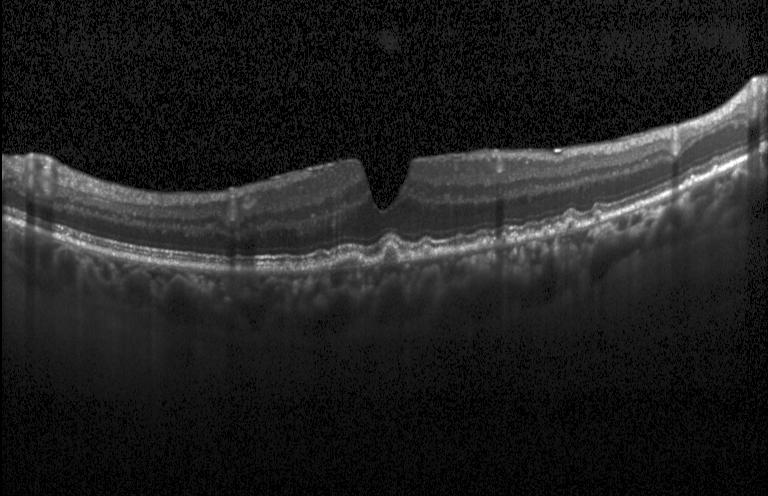
Spectral-domain OCT · Heidelberg Spectralis OCT system · optical coherence tomography B-scan · horizontal scan through the fovea.
Assessment: drusen.